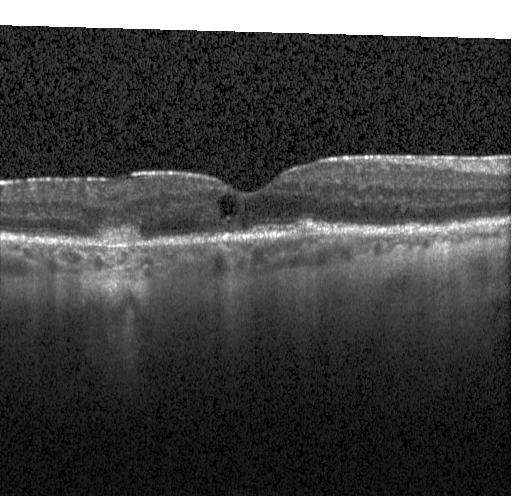

Acquired on a Heidelberg Spectralis · OCT B-scan · macular scan · spectral-domain OCT.
Impression: a choroidal neovascular membrane.